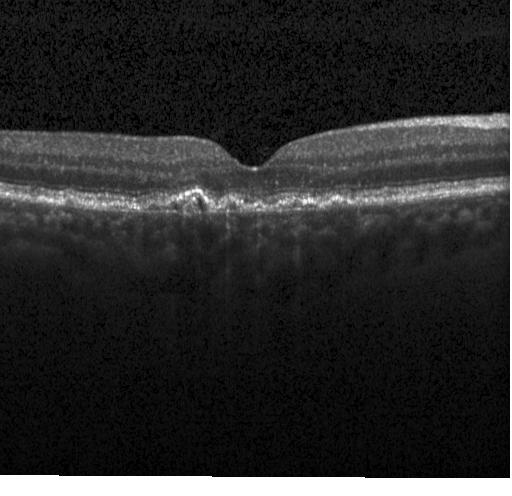

Macular OCT: a choroidal neovascular membrane.